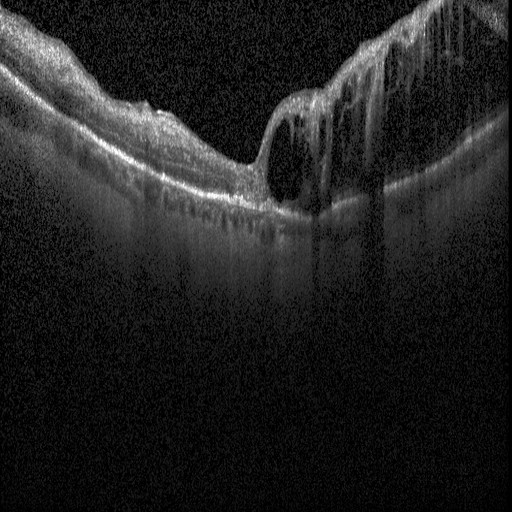 Horizontal scan through the fovea; optical coherence tomography B-scan — Assessment: diabetic macular edema (DME).